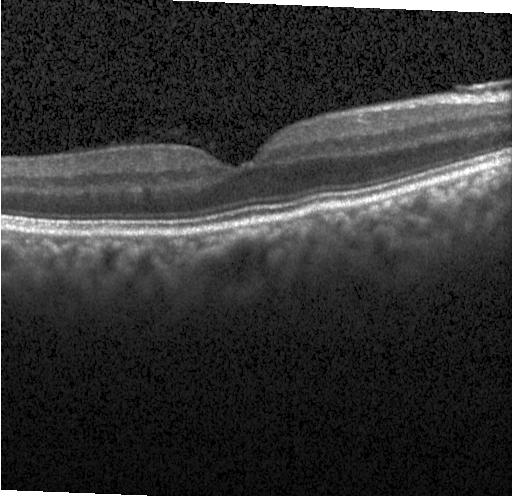 OCT B-scan
Assessment: neither choroidal neovascularization, diabetic macular edema, nor drusen.